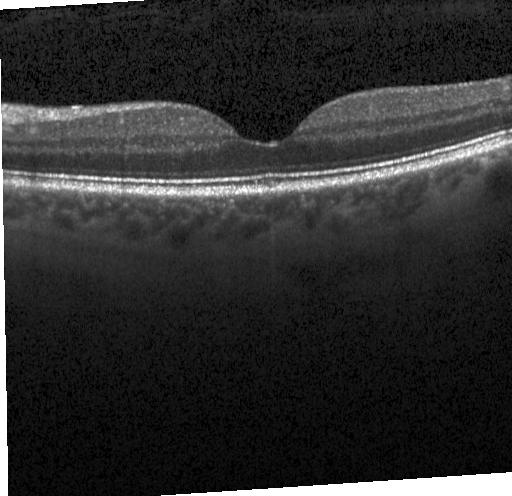 Spectral-domain optical coherence tomography. Acquired on a Heidelberg Spectralis. Centered on the fovea. Retinal OCT cross-section
No choroidal neovascularization, diabetic macular edema, or drusen.